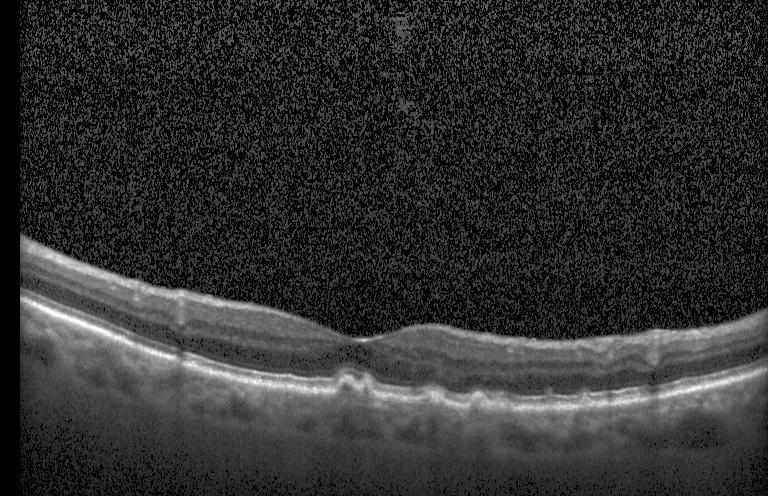
Retinal OCT cross-section — Assessment: sub-RPE drusenoid deposits.